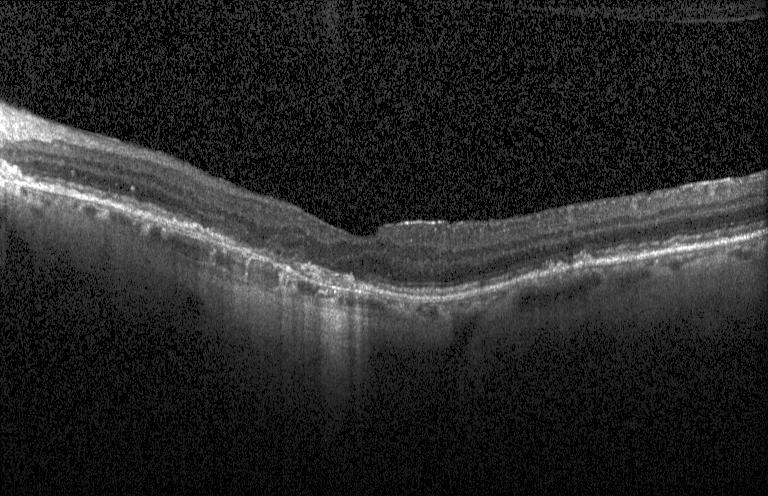
Finding: neither choroidal neovascularization, diabetic macular edema, nor drusen.